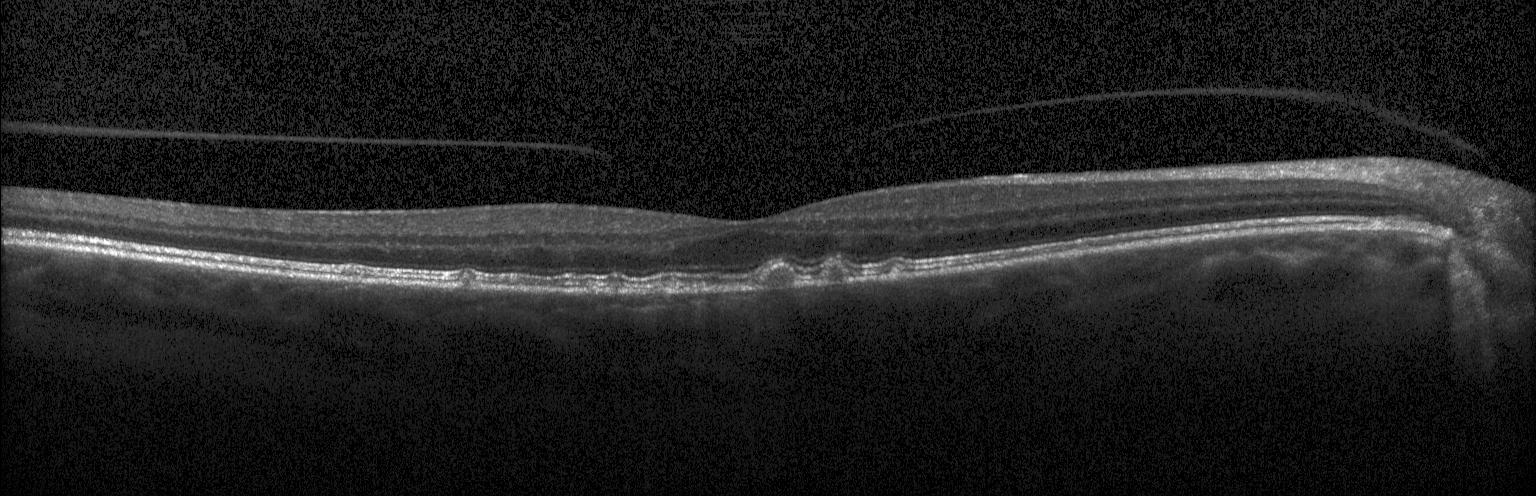 Spectral-domain optical coherence tomography. Fovea-centered. Optical coherence tomography B-scan — Multiple drusen.